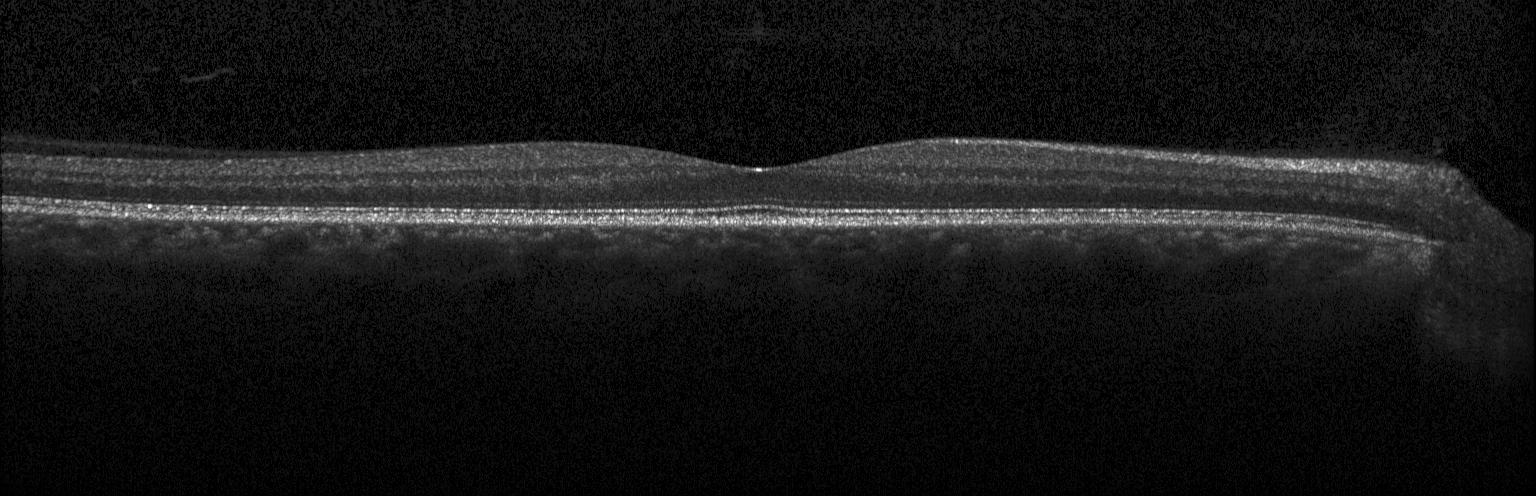

Optical coherence tomography B-scan — Impression: no CNV, no DME, and no drusen.